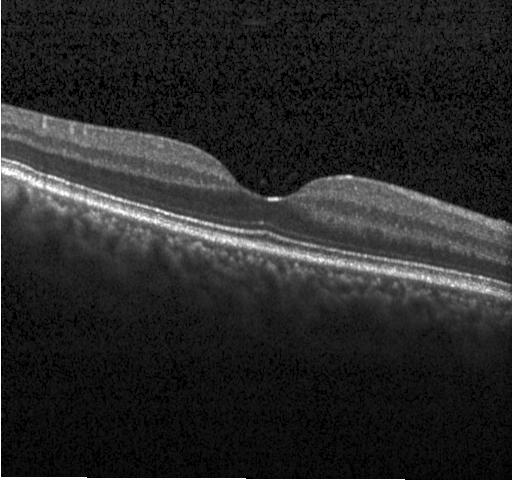

No CNV, DME, or drusen.